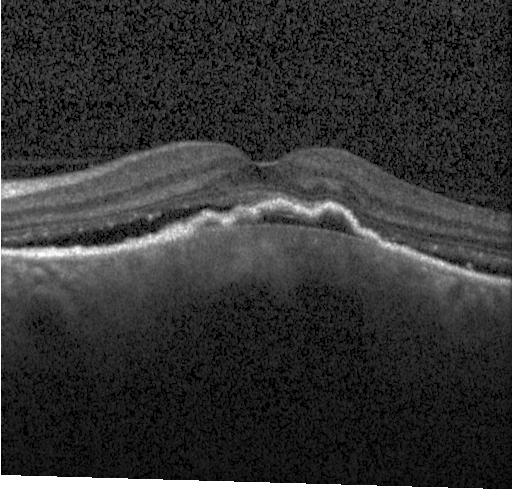
OCT B-scan. The scan shows a choroidal neovascular membrane.